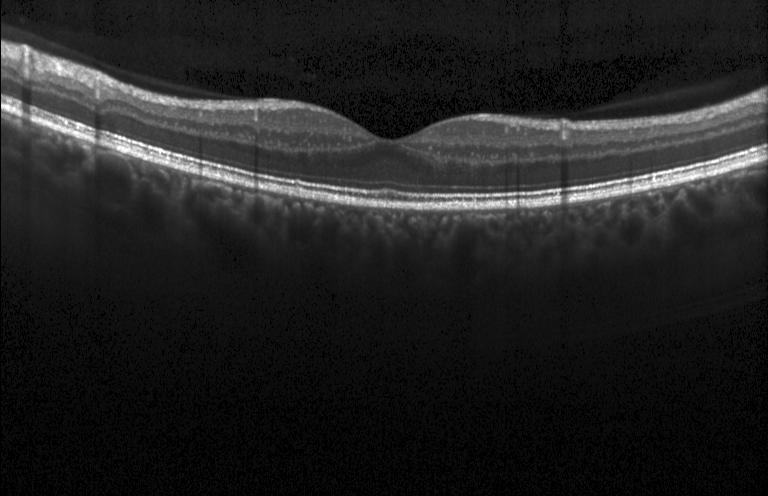 Spectral-domain optical coherence tomography. OCT line scan. Instrument: Heidelberg Spectralis — Dx: neither choroidal neovascularization, diabetic macular edema, nor drusen.